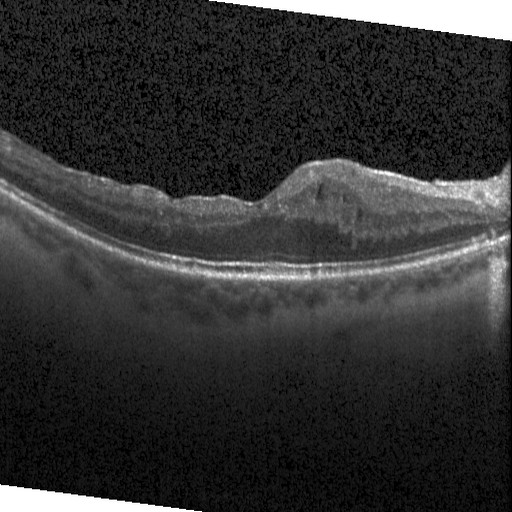
Optical coherence tomography scan
Finding: diabetic macular edema (DME).